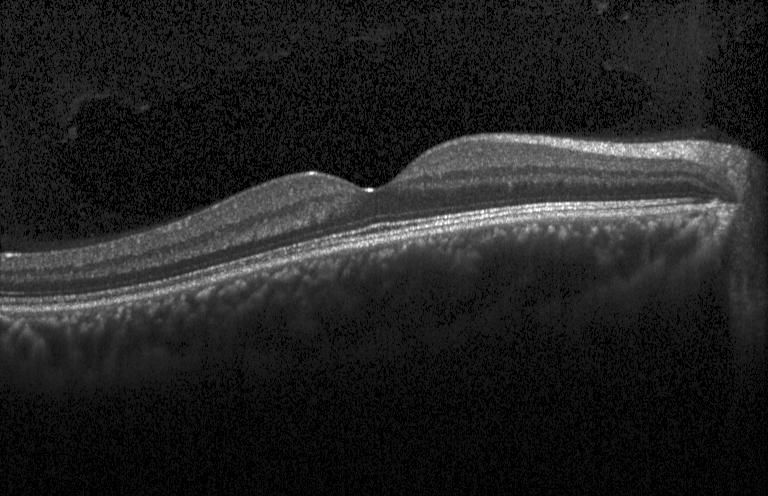
OCT B-scan; horizontal scan through the fovea.
Diagnosis: neither CNV, DME, nor drusen.